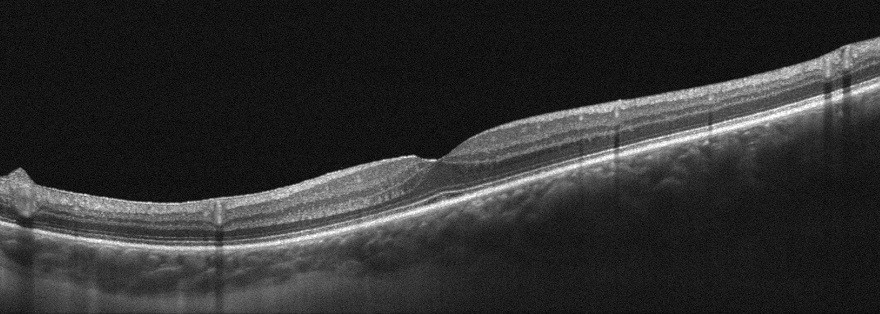 Assessment: epiretinal membrane (ERM).